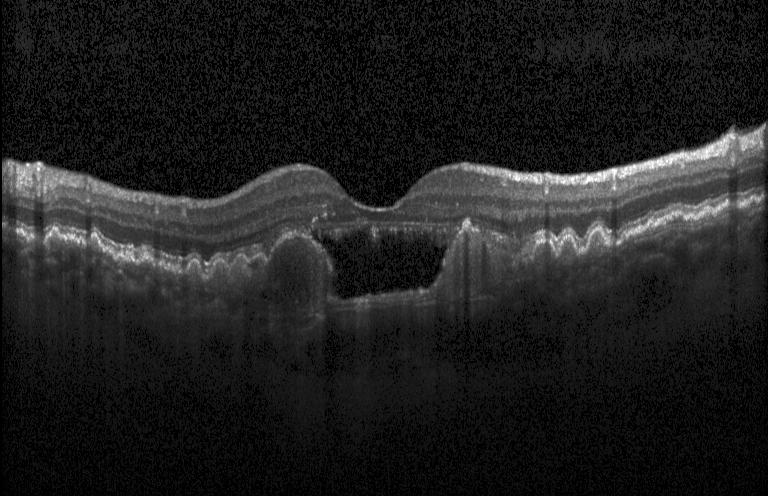 Optical coherence tomography scan — A choroidal neovascular membrane.